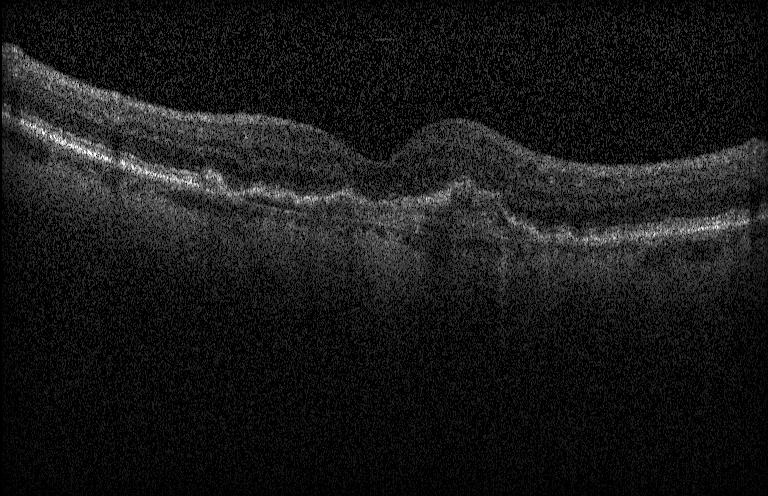 The scan shows a choroidal neovascular membrane.